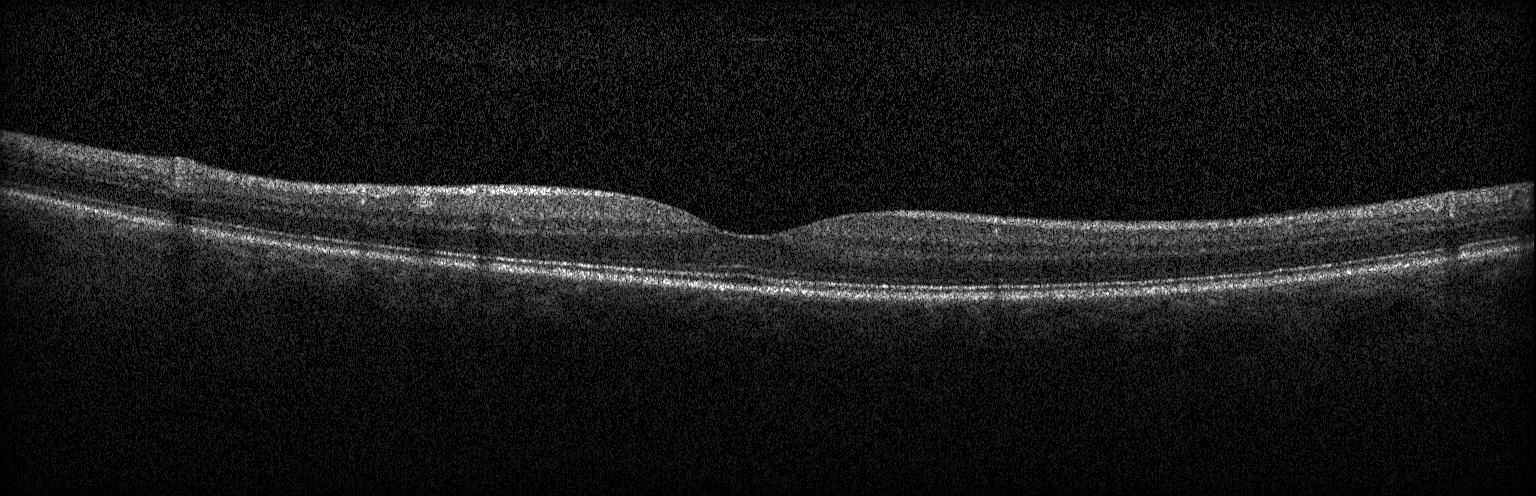

OCT scan showing neither choroidal neovascularization, diabetic macular edema, nor drusen.